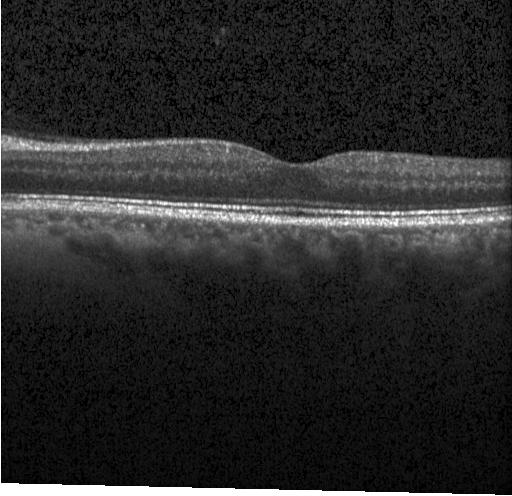
Diagnosis: no choroidal neovascularization, no diabetic macular edema, and no drusen.